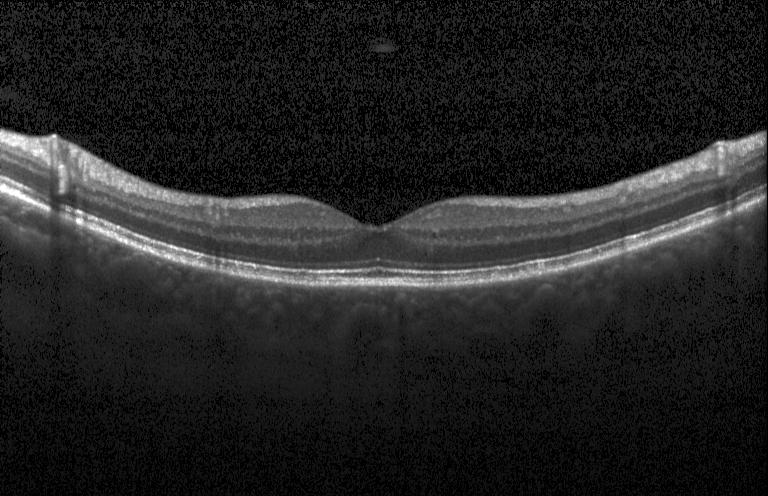
No choroidal neovascularization, diabetic macular edema, or drusen.